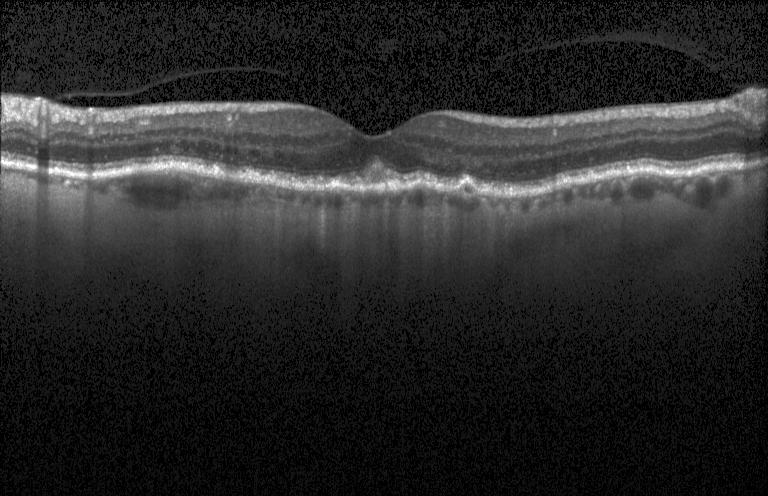
Retinal OCT B-scan; acquired on a Heidelberg Spectralis; macular scan.
This B-scan demonstrates multiple drusen.